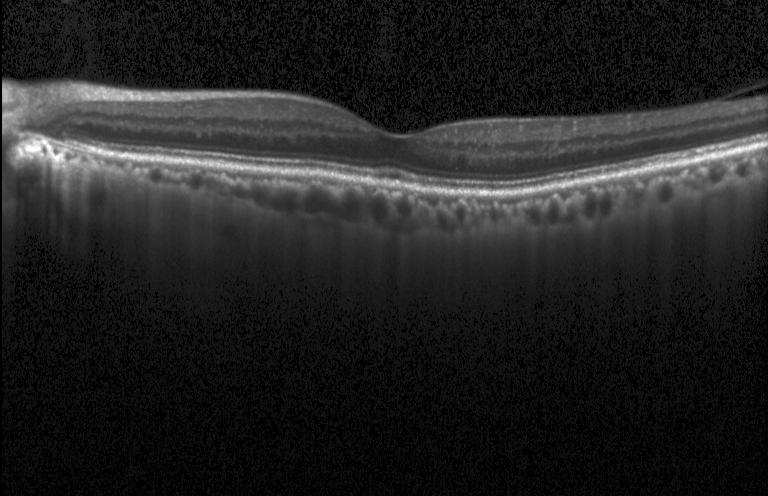 Retinal OCT B-scan. Acquired on a Heidelberg Spectralis. Spectral-domain optical coherence tomography. Horizontal scan through the fovea
Impression: no choroidal neovascularization, diabetic macular edema, or drusen.